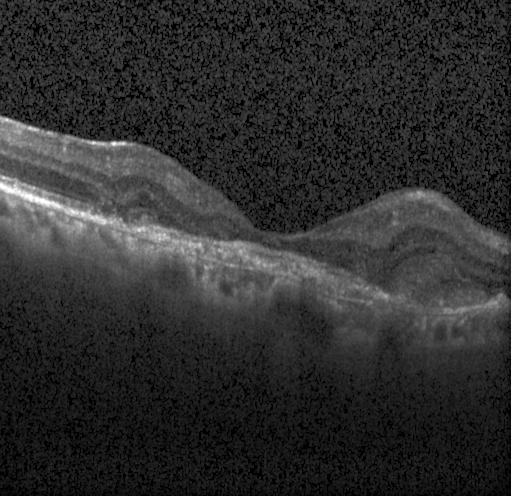 Optical coherence tomography B-scan
The scan shows a choroidal neovascular membrane.